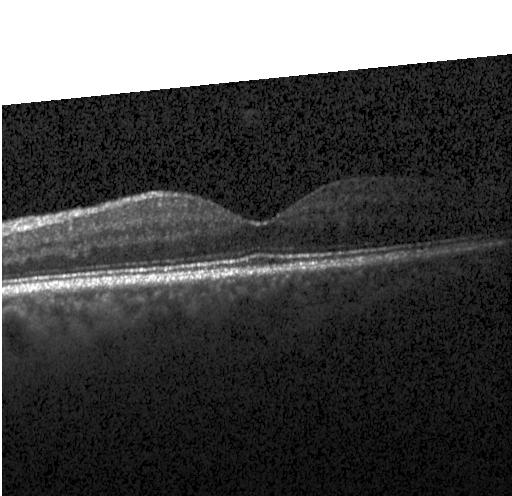

Macular OCT: neither choroidal neovascularization, diabetic macular edema, nor drusen.